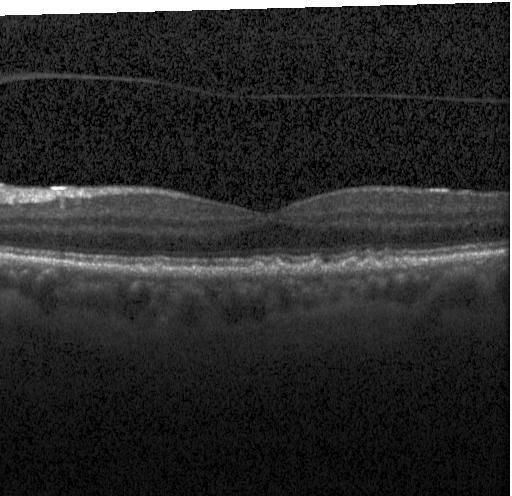 Instrument: Heidelberg Spectralis · retinal OCT cross-section · macular scan.
The scan shows sub-RPE drusenoid deposits.